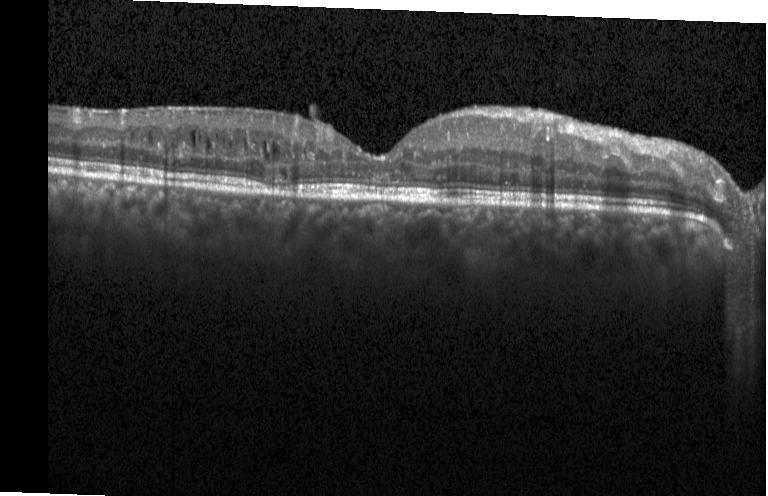

Retinal OCT cross-section
The scan shows diabetic macular edema.